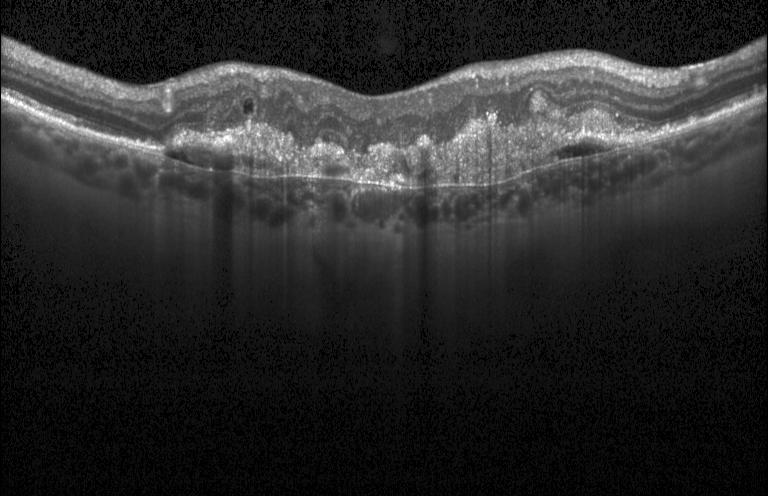

Retinal OCT cross-section.
Dx: choroidal neovascularization (CNV).